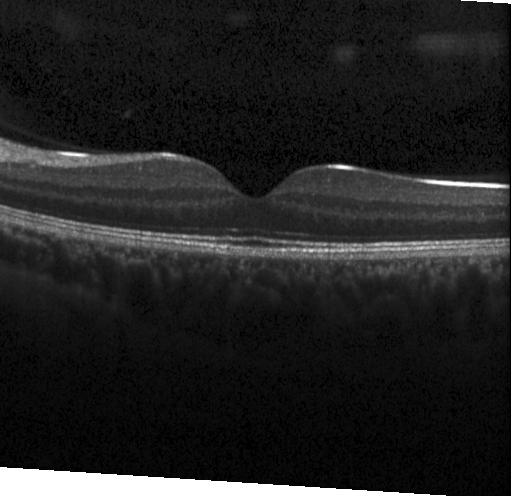
OCT B-scan. OCT finding: no choroidal neovascularization, diabetic macular edema, or drusen.